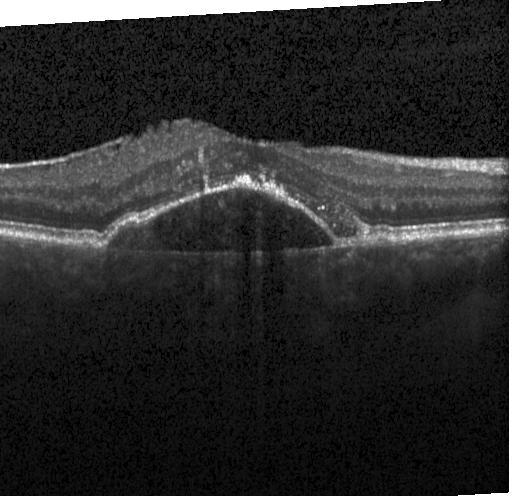
Finding: a choroidal neovascular membrane.